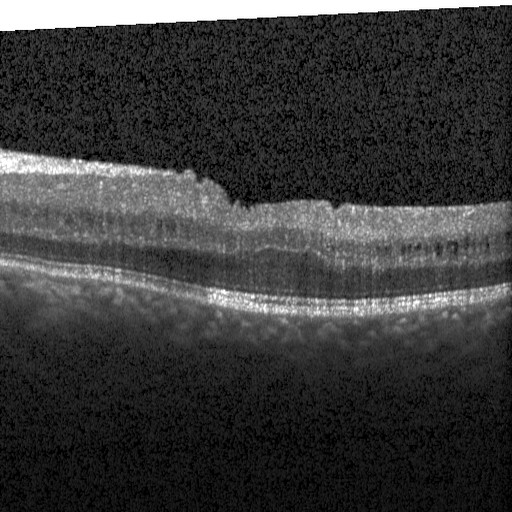
Spectral-domain OCT, horizontal scan through the fovea, optical coherence tomography scan.
Diagnosis: DME.